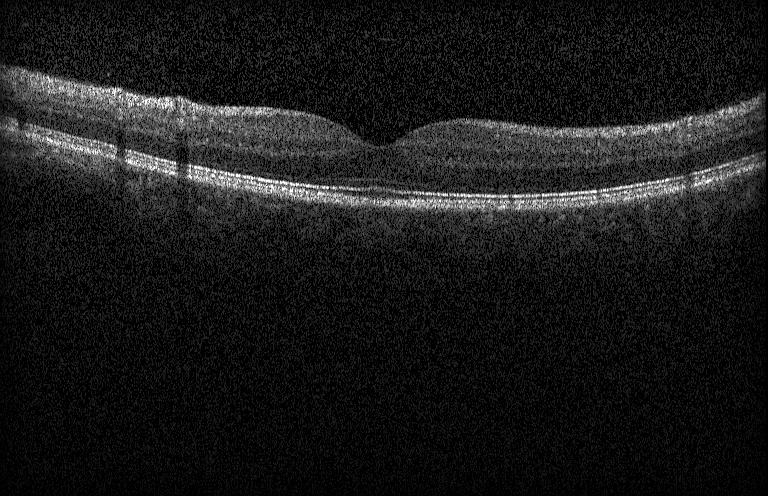

OCT line scan
Impression: neither choroidal neovascularization, diabetic macular edema, nor drusen.